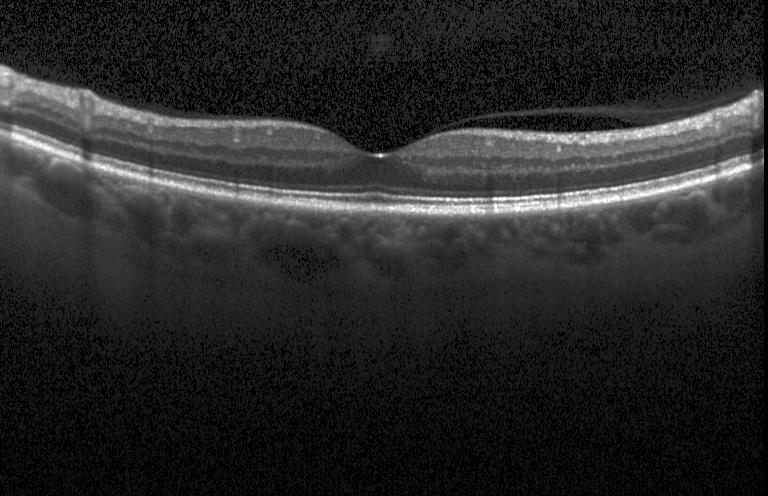 OCT finding: no choroidal neovascularization, diabetic macular edema, or drusen.